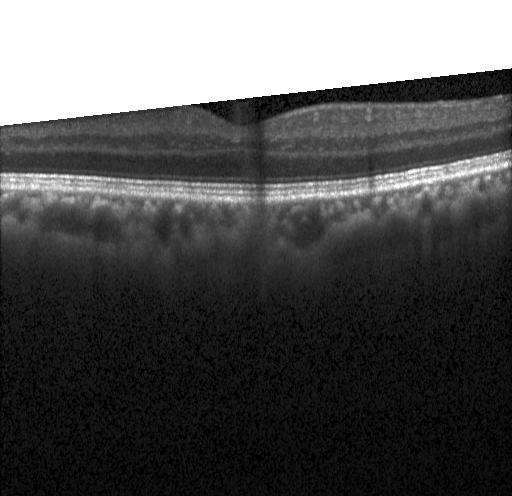
The scan shows no CNV, no DME, and no drusen.